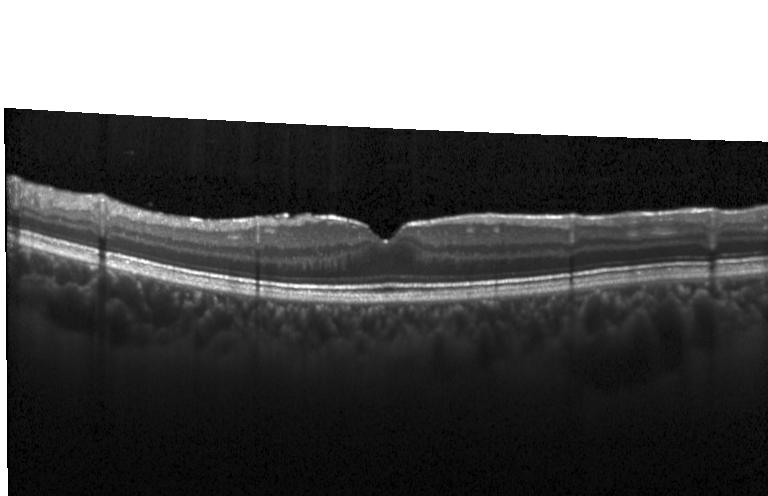 OCT finding: no CNV, no DME, and no drusen.